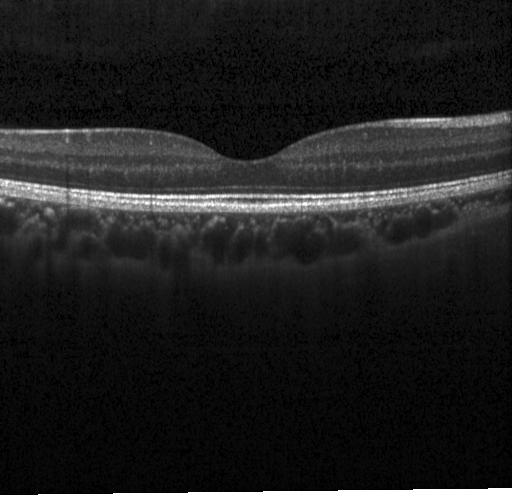
OCT line scan. Diagnosis: no choroidal neovascularization, no diabetic macular edema, and no drusen.